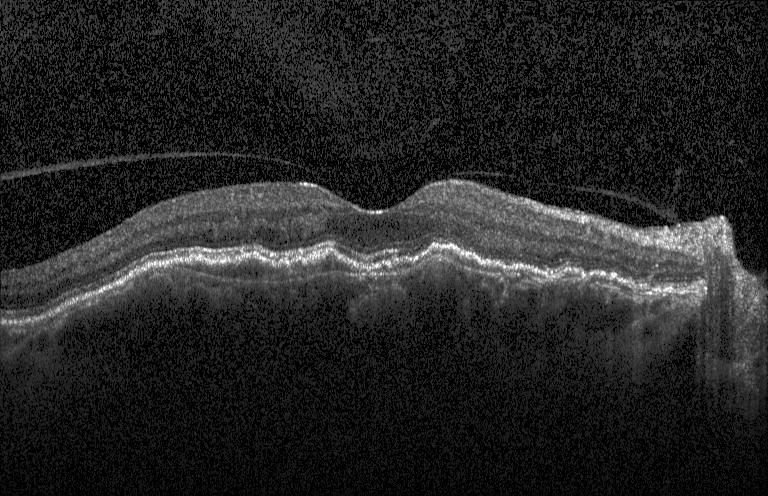

Instrument: Heidelberg Spectralis. OCT B-scan — Finding: a choroidal neovascular membrane.